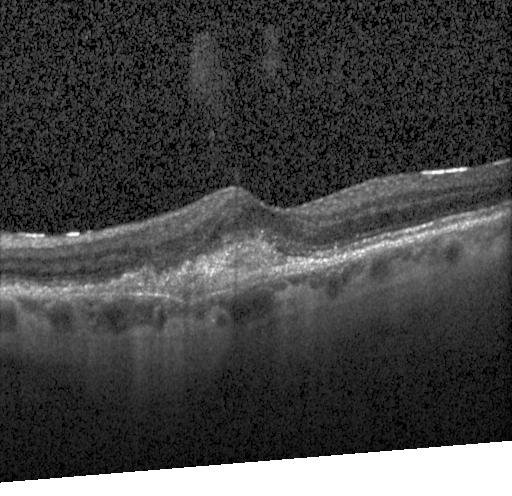

OCT finding: a choroidal neovascular membrane.